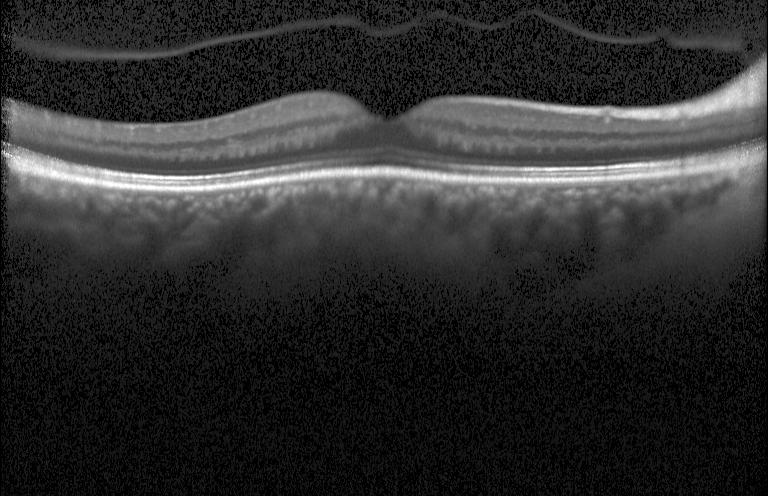

Through the macula, retinal OCT B-scan.
OCT finding: no evidence of choroidal neovascularization, diabetic macular edema, or drusen.